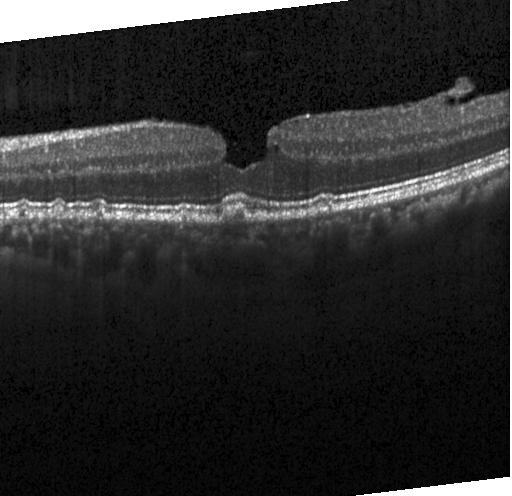 Finding: multiple drusen.